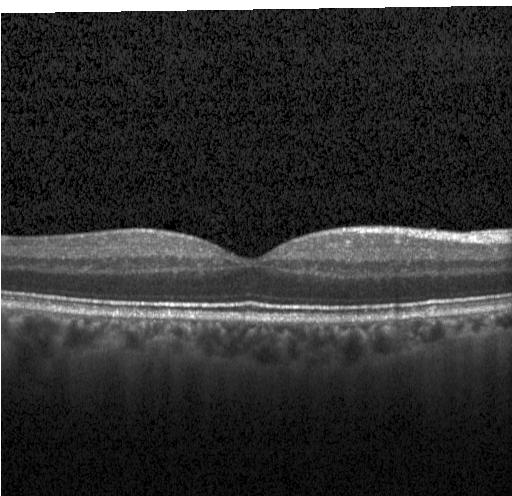 Finding: no CNV, DME, or drusen.